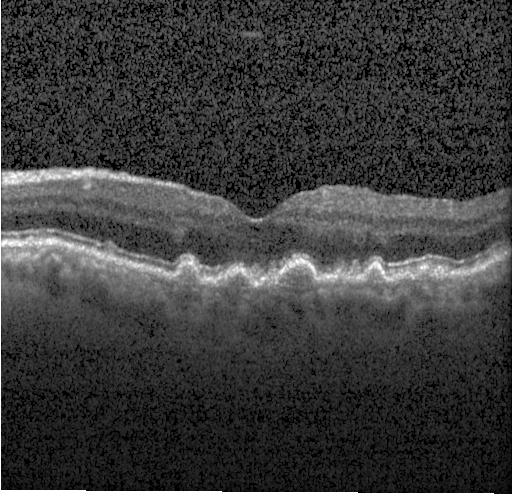

Spectral-domain OCT B-scan: sub-RPE drusenoid deposits.